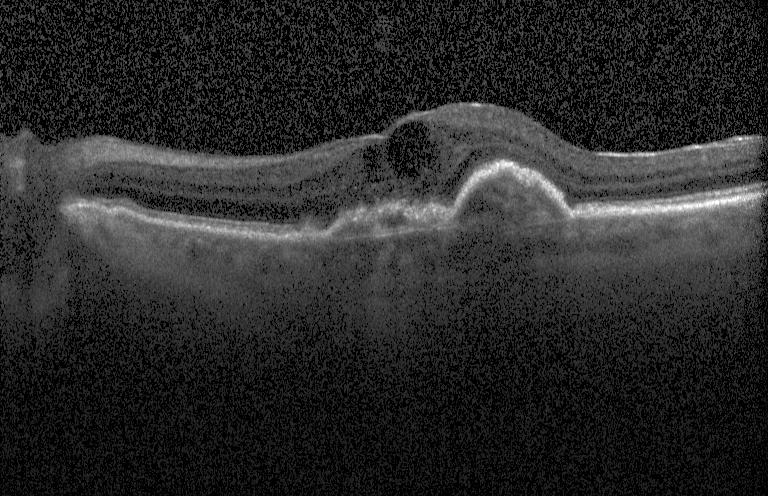 Spectral-domain OCT · Heidelberg Spectralis OCT system · fovea-centered · retinal OCT B-scan. Finding: a choroidal neovascular membrane.